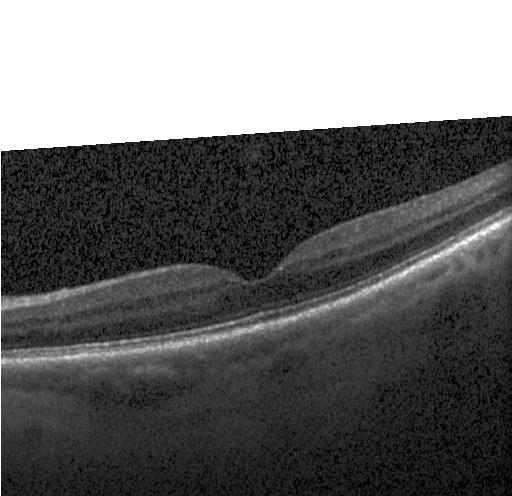
Retinal OCT cross-section — Assessment: no choroidal neovascularization, no diabetic macular edema, and no drusen.